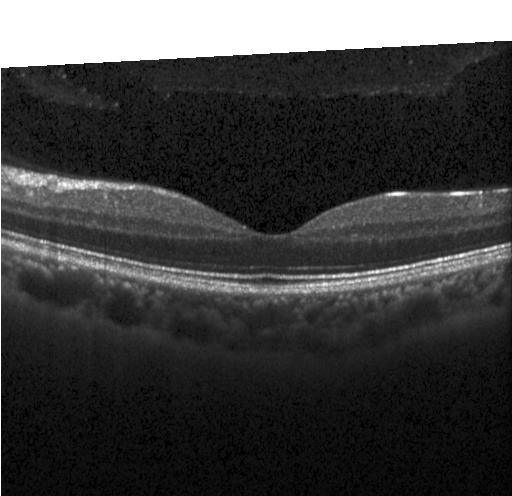

Through the macula, SD-OCT, optical coherence tomography scan. Finding: no choroidal neovascularization, diabetic macular edema, or drusen.